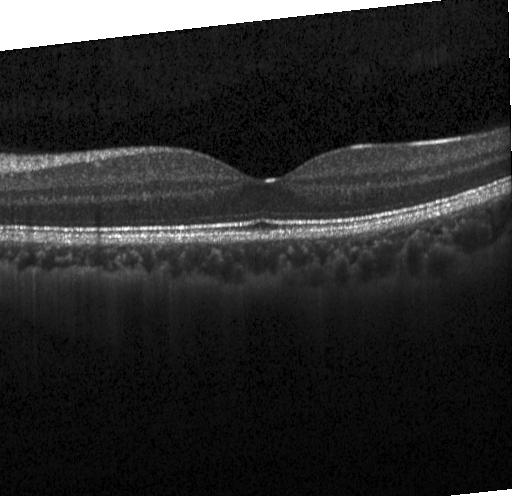 Retinal OCT B-scan — Diagnosis: no evidence of choroidal neovascularization, diabetic macular edema, or drusen.